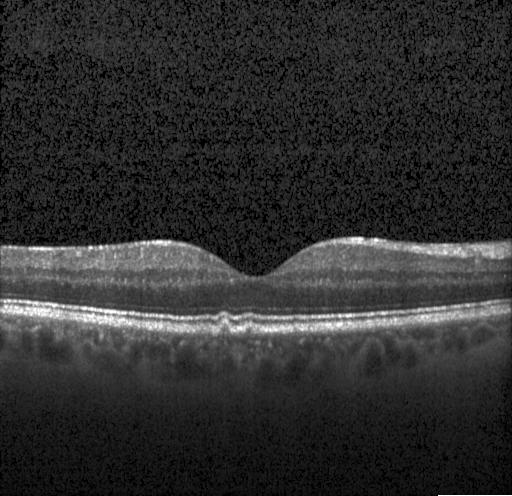 SD-OCT; retinal OCT B-scan; Heidelberg Spectralis
Sub-RPE drusenoid deposits.